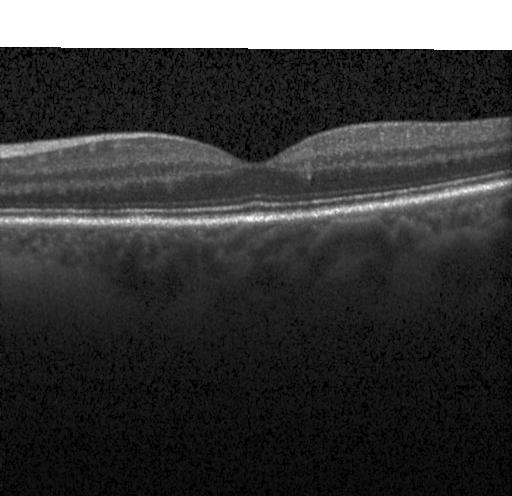
OCT line scan, horizontal scan through the fovea, spectral-domain optical coherence tomography, Heidelberg Spectralis. The scan shows no CNV, DME, or drusen.